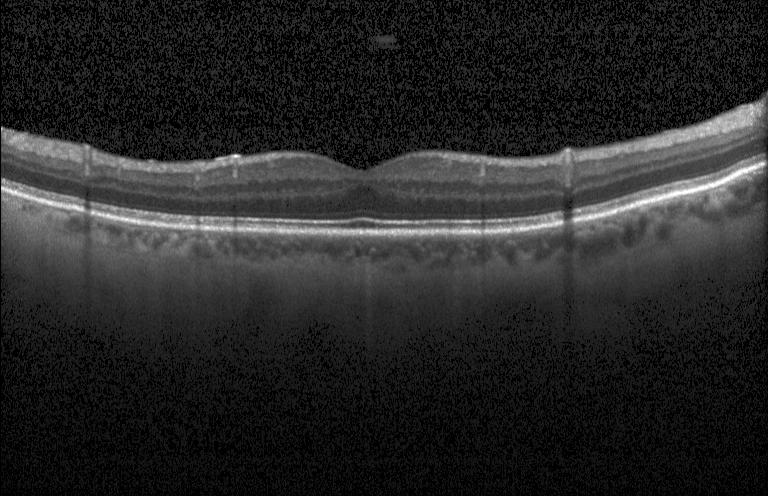 Retinal OCT cross-section.
Finding: no evidence of choroidal neovascularization, diabetic macular edema, or drusen.